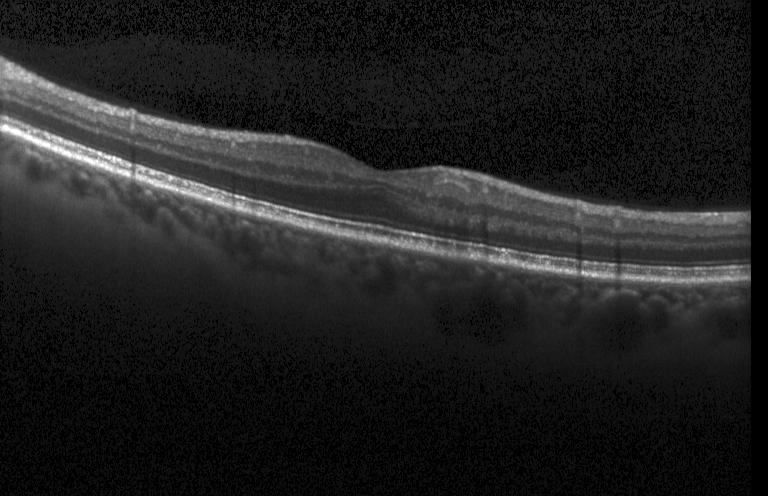 Acquired on a Heidelberg Spectralis; fovea-centered; OCT B-scan. Assessment: no choroidal neovascularization, no diabetic macular edema, and no drusen.